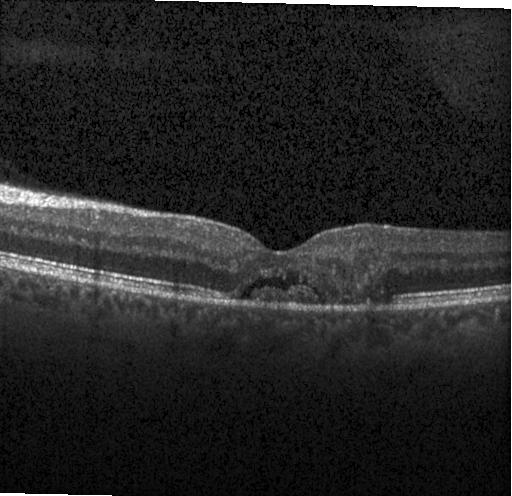 OCT line scan.
Finding: a choroidal neovascular membrane.